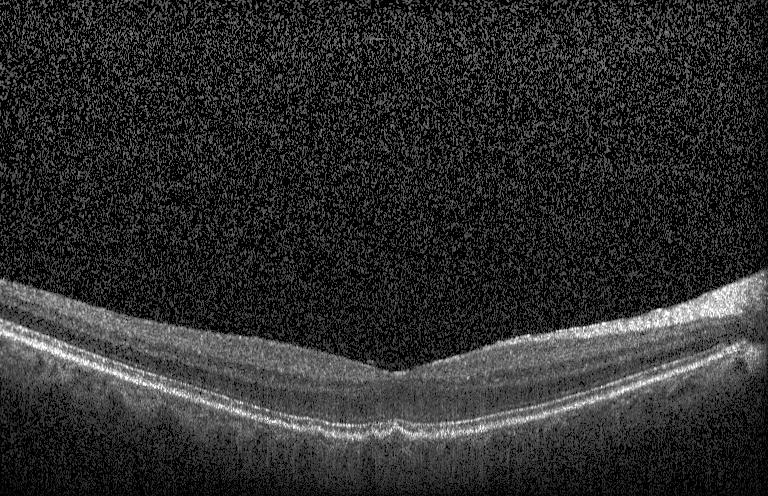 Spectral-domain optical coherence tomography, OCT line scan.
Diagnosis: sub-RPE drusenoid deposits.